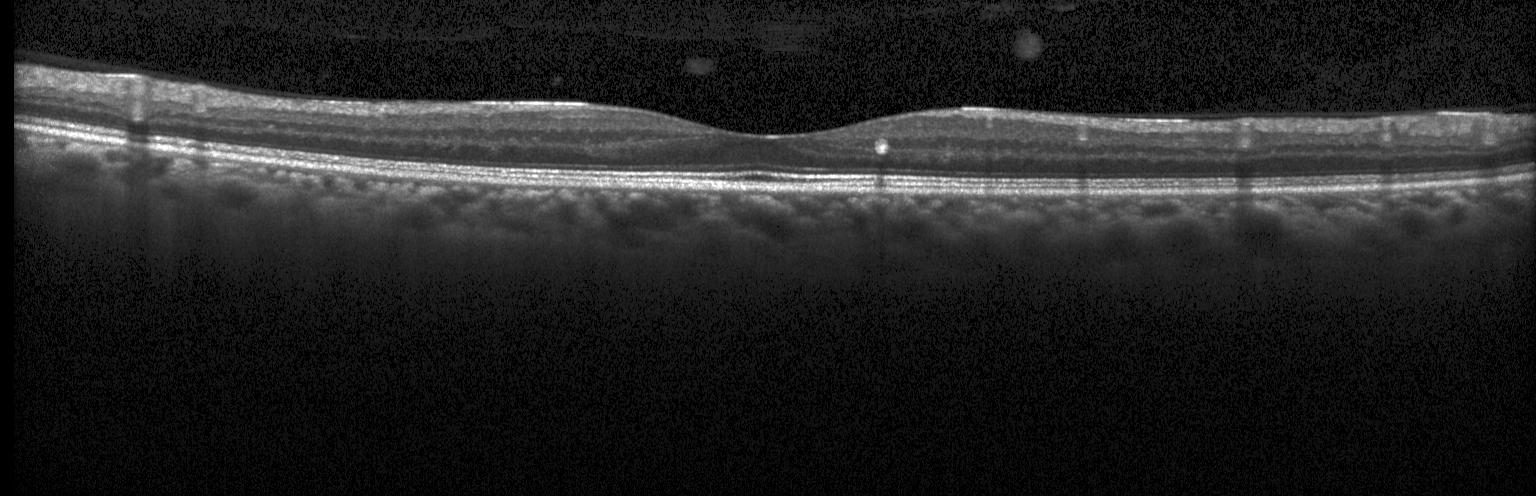 Retinal OCT cross-section; acquired on a Heidelberg Spectralis; centered on the fovea.
Assessment: neither CNV, DME, nor drusen.